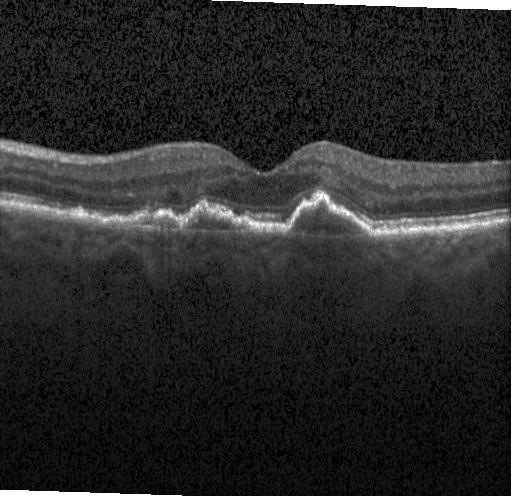
CNV.